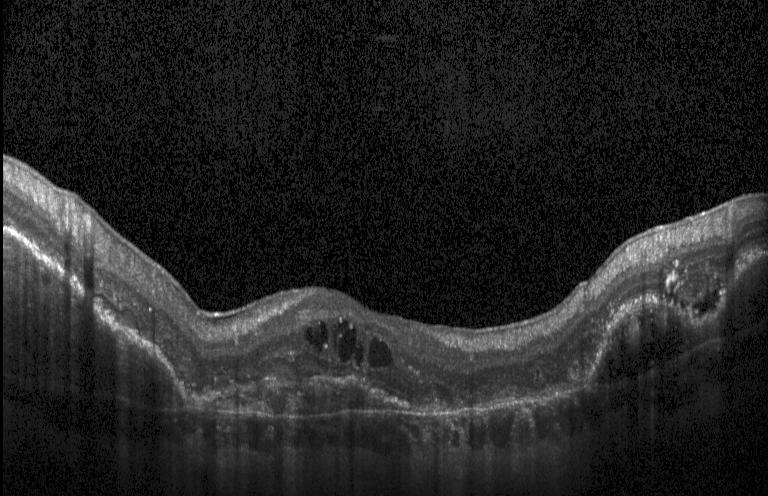

Dx: CNV.